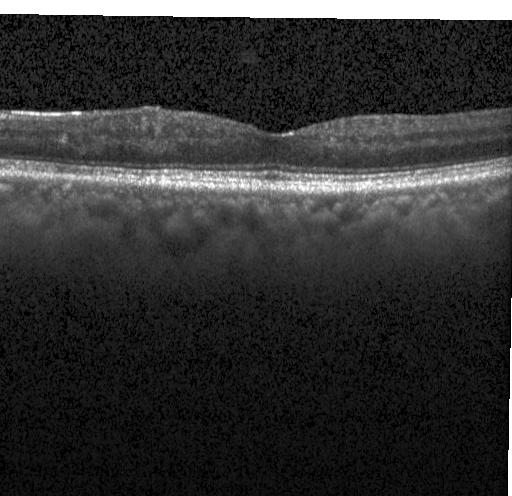 Dx: no CNV, no DME, and no drusen.